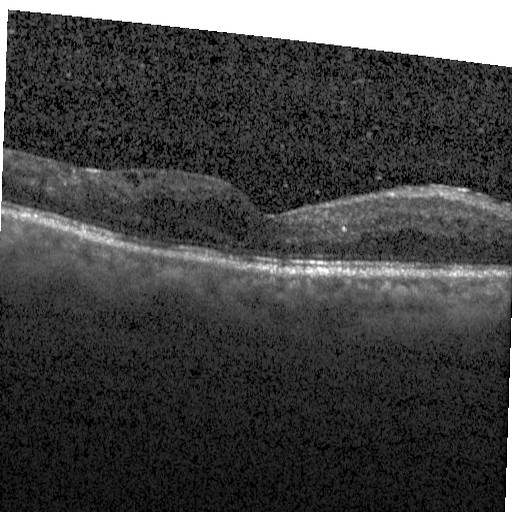 OCT line scan · spectral-domain OCT · instrument: Heidelberg Spectralis. Macular OCT: diabetic macular edema.